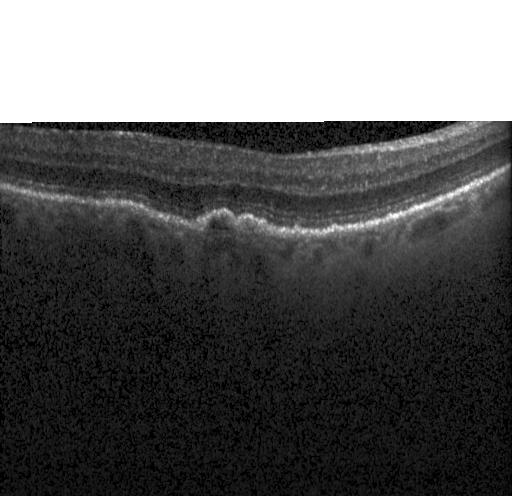 Horizontal scan through the fovea; OCT B-scan; Heidelberg Spectralis
Impression: multiple drusen.